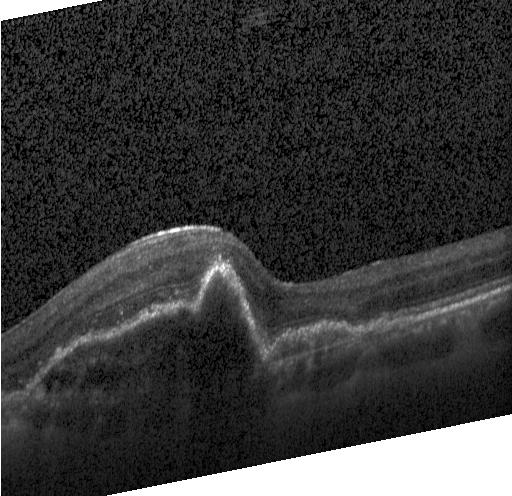 OCT scan showing a choroidal neovascular membrane.